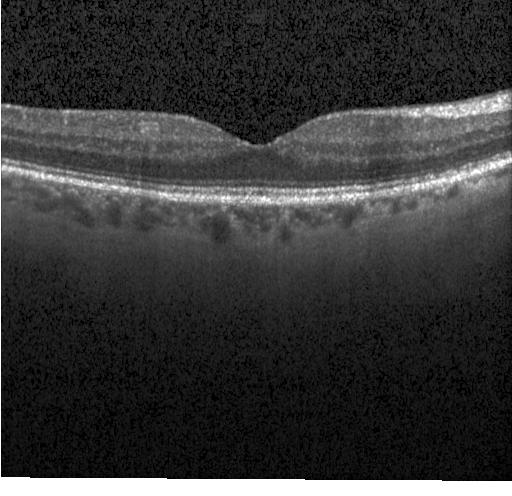 Diagnosis: neither choroidal neovascularization, diabetic macular edema, nor drusen.